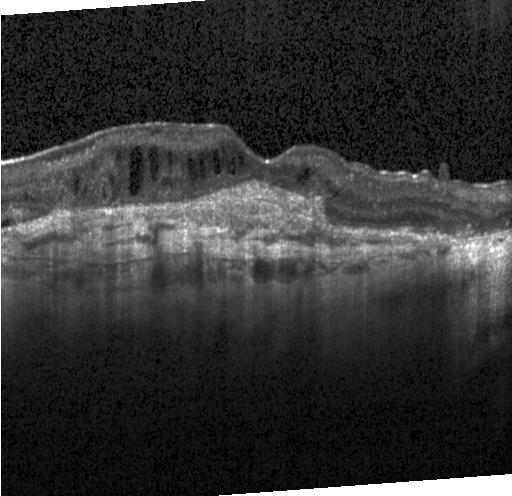 Optical coherence tomography B-scan · spectral-domain optical coherence tomography · Heidelberg Spectralis OCT system.
Assessment: CNV.